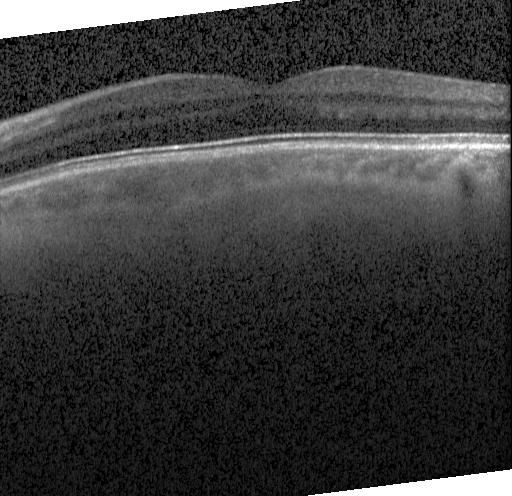
Retinal OCT cross-section
Assessment: no choroidal neovascularization, no diabetic macular edema, and no drusen.